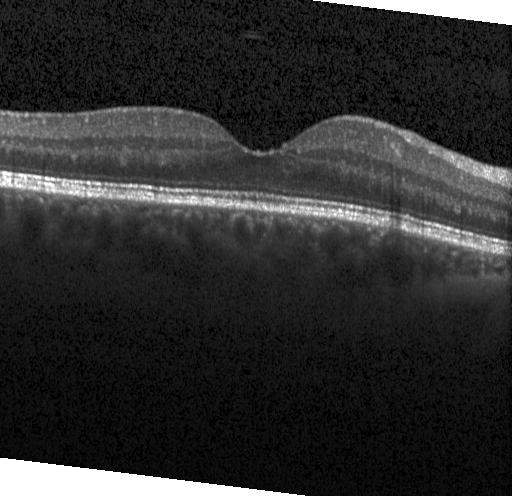
Finding: no evidence of CNV, DME, or drusen.